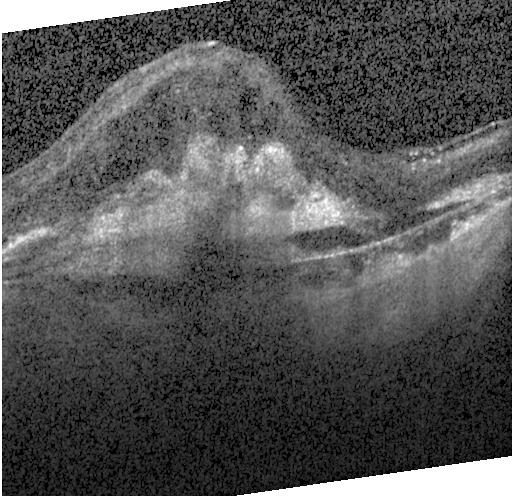
Fovea-centered, optical coherence tomography B-scan.
Assessment: choroidal neovascularization (CNV).